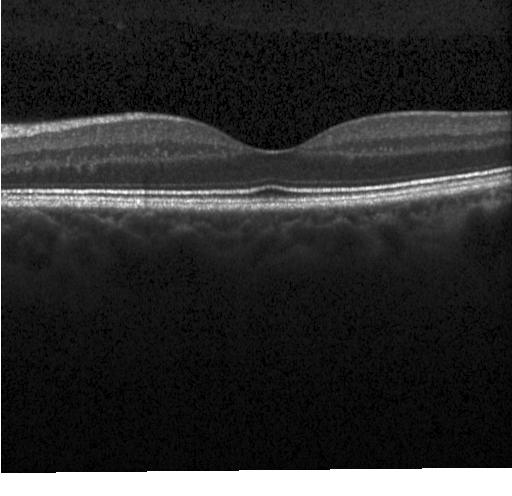 Macular scan · spectral-domain optical coherence tomography · OCT B-scan. Diagnosis: neither CNV, DME, nor drusen.